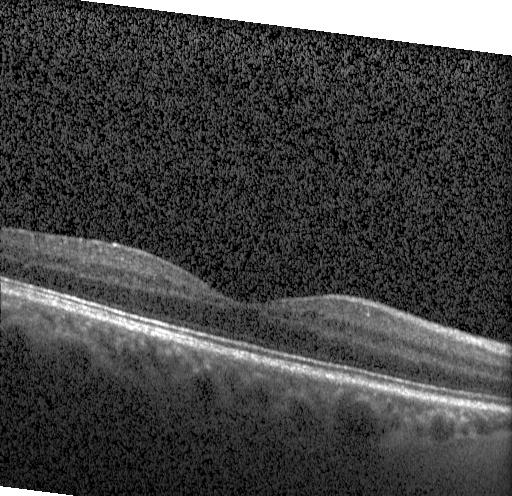
Optical coherence tomography scan. Heidelberg Spectralis. Spectral-domain OCT — Impression: no choroidal neovascularization, diabetic macular edema, or drusen.